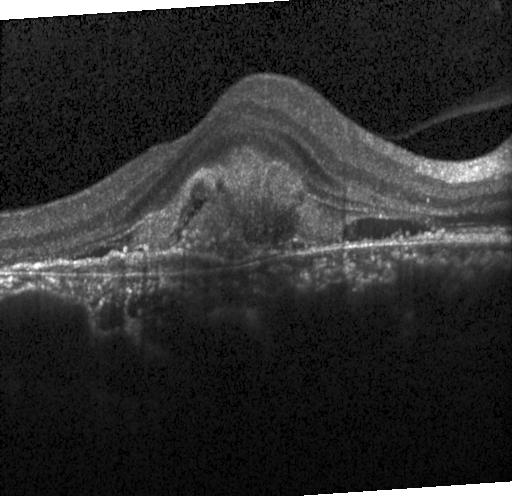 OCT line scan. Choroidal neovascularization (CNV).